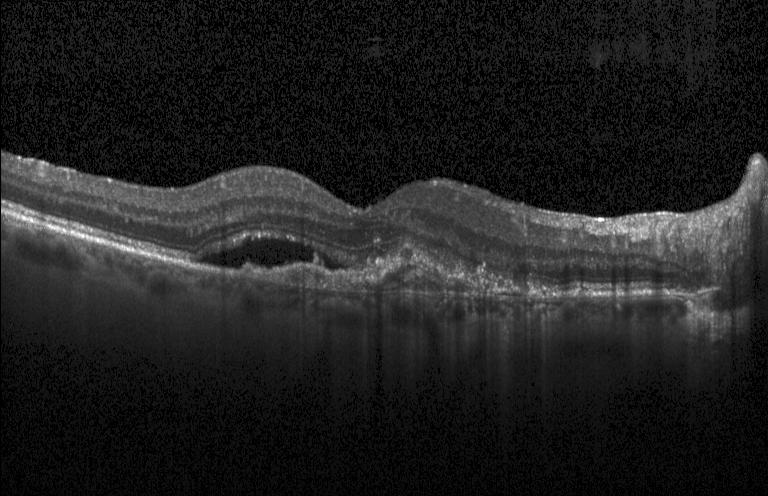 Impression: choroidal neovascularization.